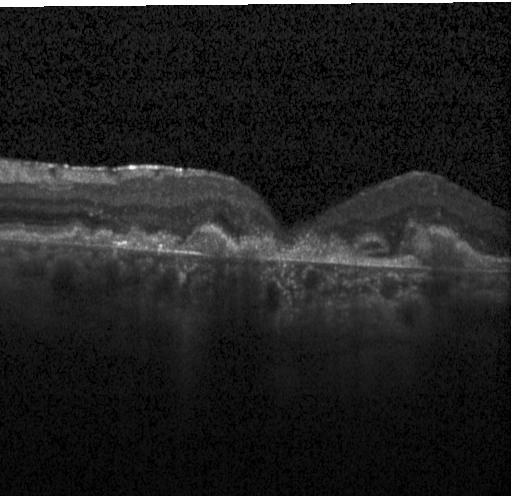
Through the macula; Heidelberg Spectralis OCT system; SD-OCT; optical coherence tomography scan
Diagnosis: a choroidal neovascular membrane.